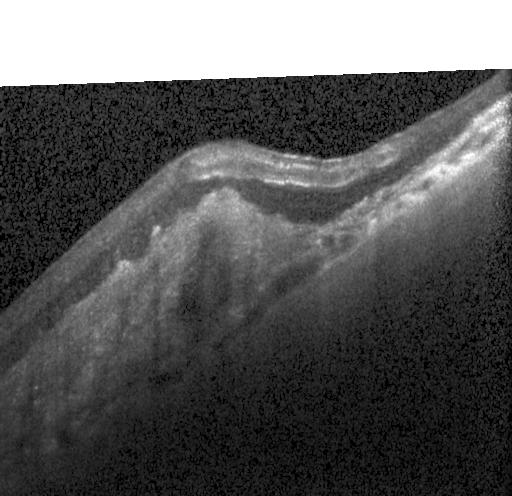 Retinal OCT cross-section — Assessment: choroidal neovascularization.